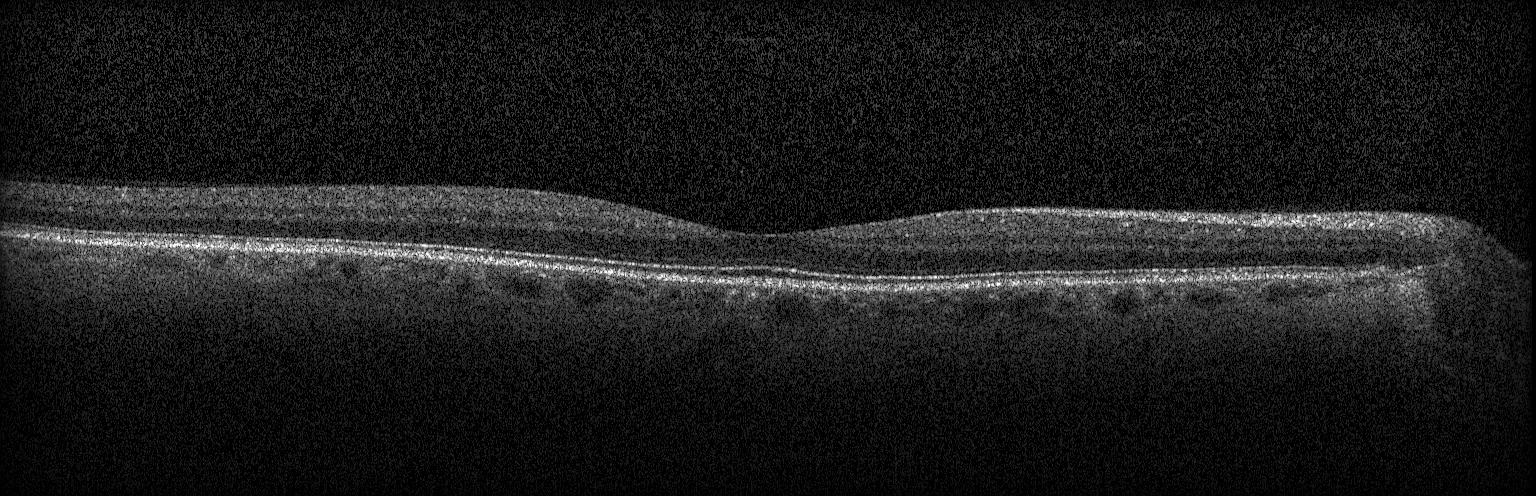

Spectral-domain OCT. Heidelberg Spectralis. Optical coherence tomography B-scan.
Finding: no evidence of choroidal neovascularization, diabetic macular edema, or drusen.